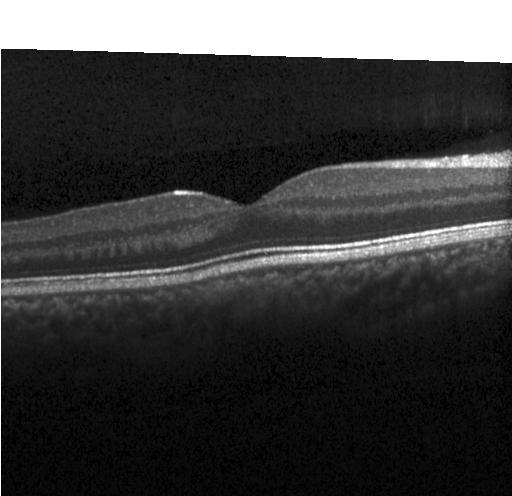

Spectral-domain optical coherence tomography. Instrument: Heidelberg Spectralis. Macular scan. OCT B-scan
OCT finding: no evidence of choroidal neovascularization, diabetic macular edema, or drusen.